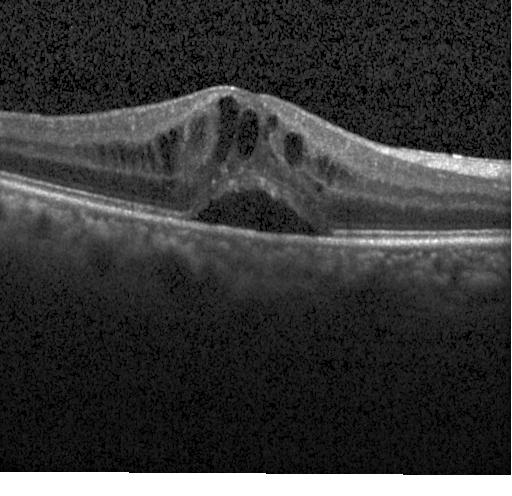

Assessment: DME.